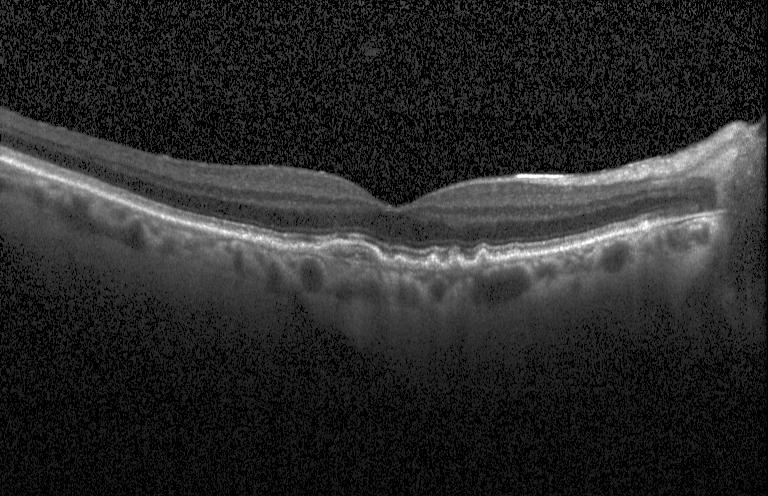

OCT finding: a choroidal neovascular membrane.